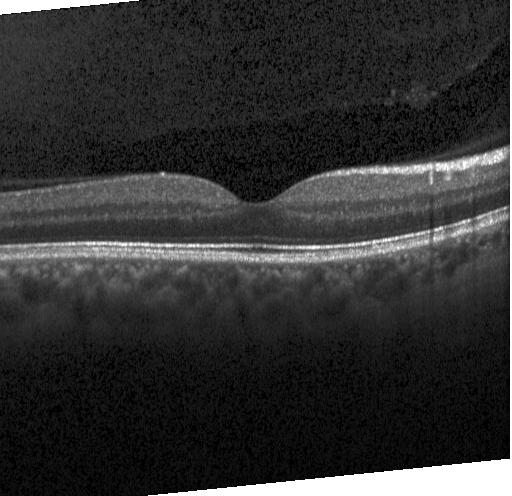
Spectral-domain optical coherence tomography, Heidelberg Spectralis, retinal OCT cross-section. Diagnosis: no choroidal neovascularization, diabetic macular edema, or drusen.